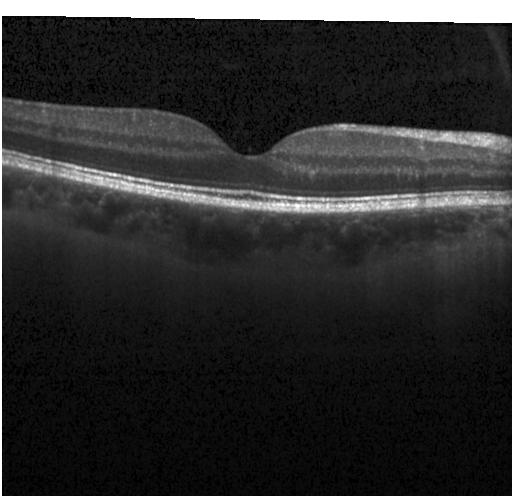 OCT finding: no evidence of CNV, DME, or drusen.